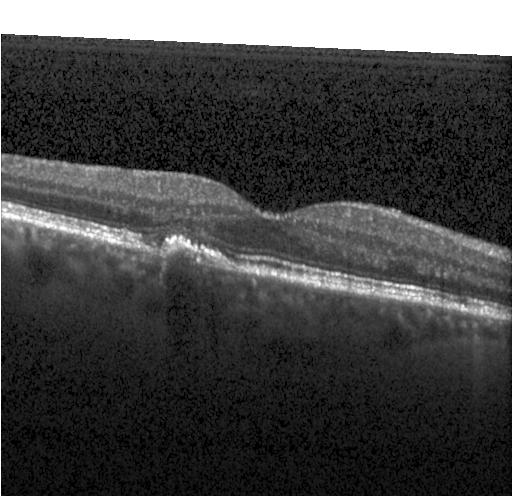
A choroidal neovascular membrane.